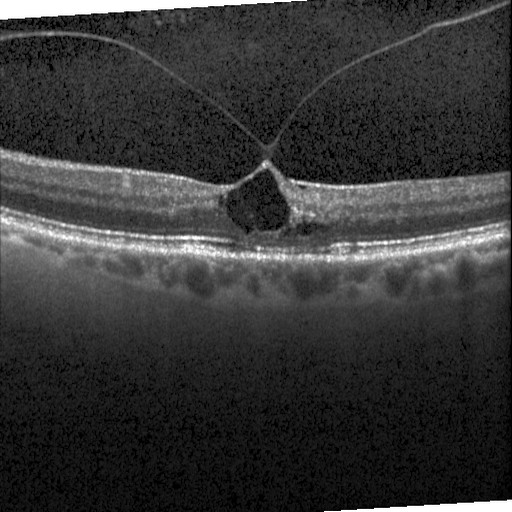
OCT B-scan; spectral-domain OCT.
Diagnosis: diabetic macular edema.